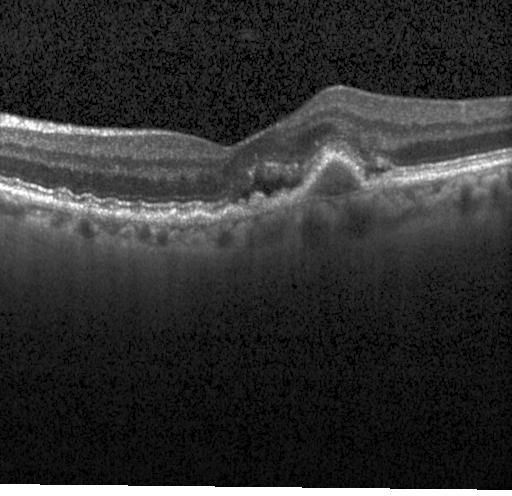

SD-OCT; OCT B-scan.
Choroidal neovascularization (CNV).